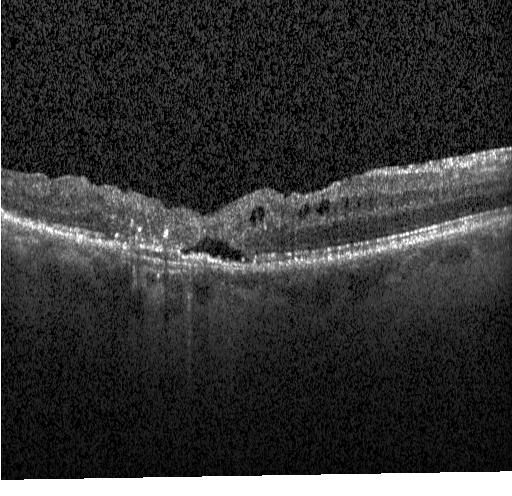 Optical coherence tomography B-scan. Impression: a choroidal neovascular membrane.